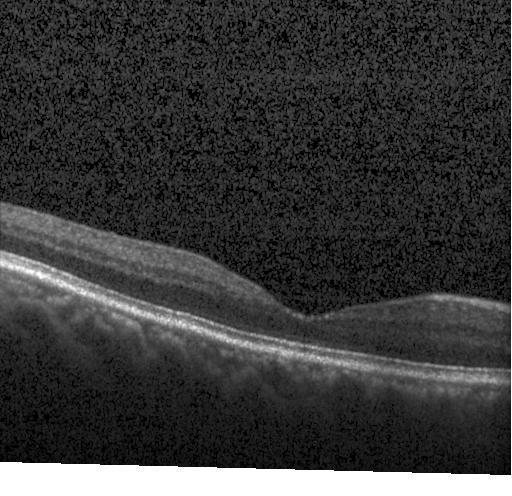

Impression: no choroidal neovascularization, no diabetic macular edema, and no drusen.